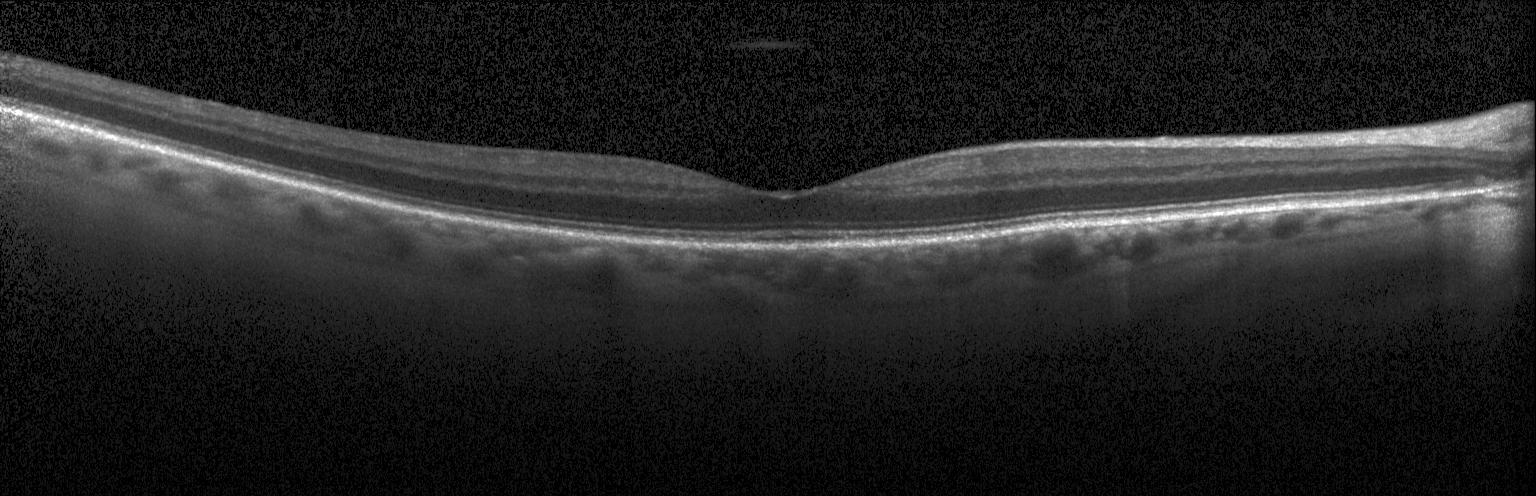
SD-OCT, OCT B-scan, acquired on a Heidelberg Spectralis, through the macula — Dx: no choroidal neovascularization, diabetic macular edema, or drusen.